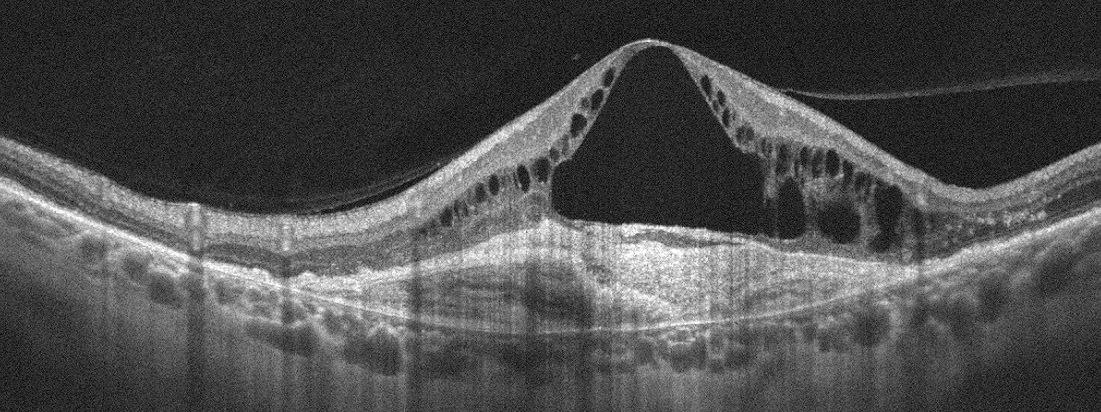

Retinal OCT cross-section showing age-related macular degeneration (AMD).